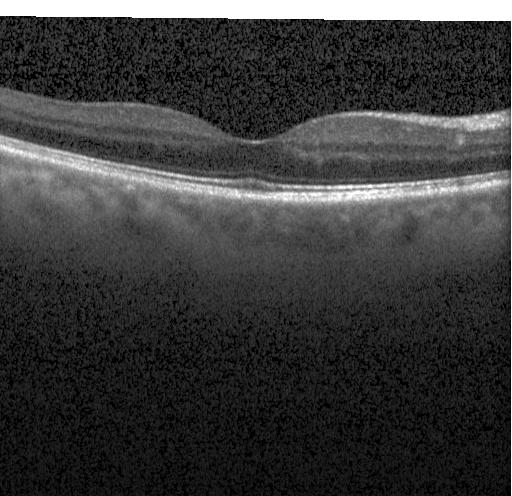

Finding: neither choroidal neovascularization, diabetic macular edema, nor drusen.